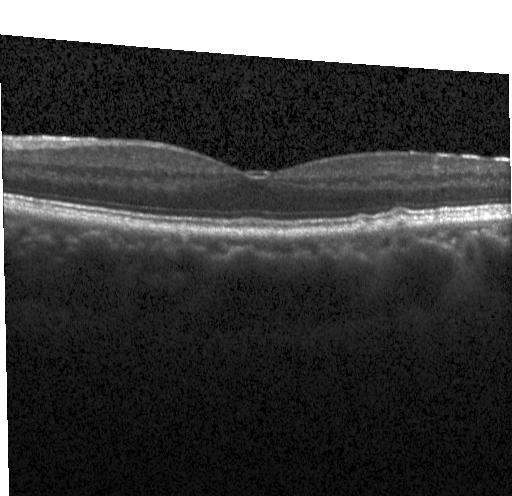

OCT line scan.
Finding: drusen.